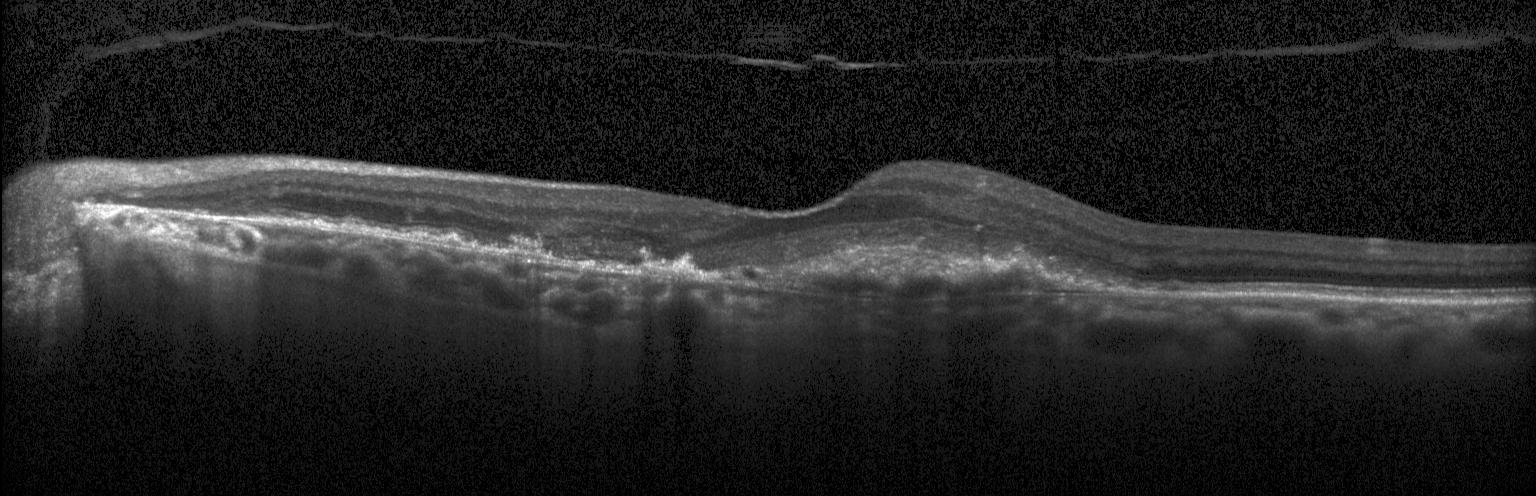
OCT line scan · Heidelberg Spectralis. Finding: choroidal neovascularization (CNV).